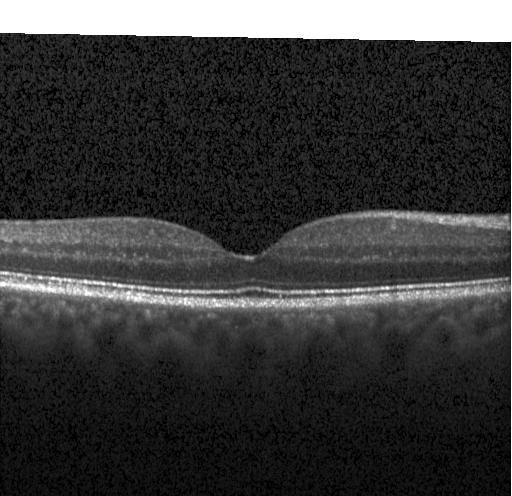

This B-scan demonstrates neither choroidal neovascularization, diabetic macular edema, nor drusen.